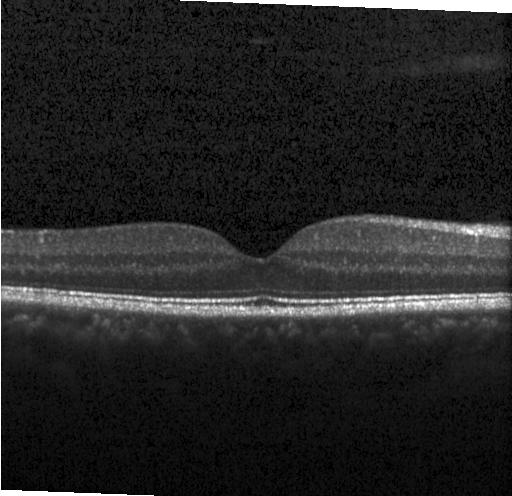 Retinal OCT cross-section showing no CNV, DME, or drusen.